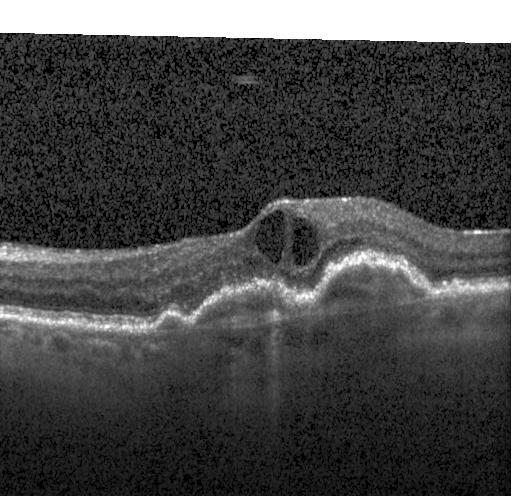 Impression: choroidal neovascularization (CNV).